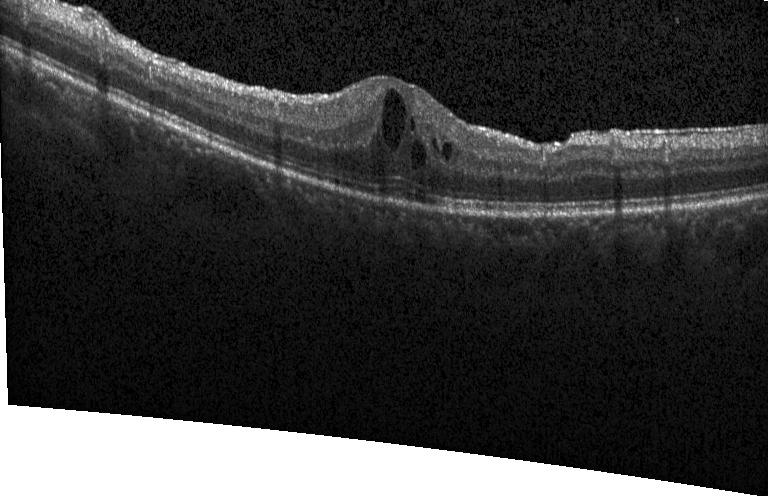

Retinal OCT B-scan. Finding: DME.